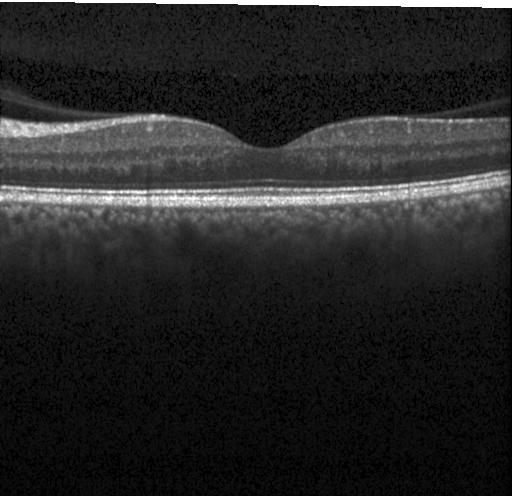

Optical coherence tomography B-scan.
Diagnosis: neither choroidal neovascularization, diabetic macular edema, nor drusen.